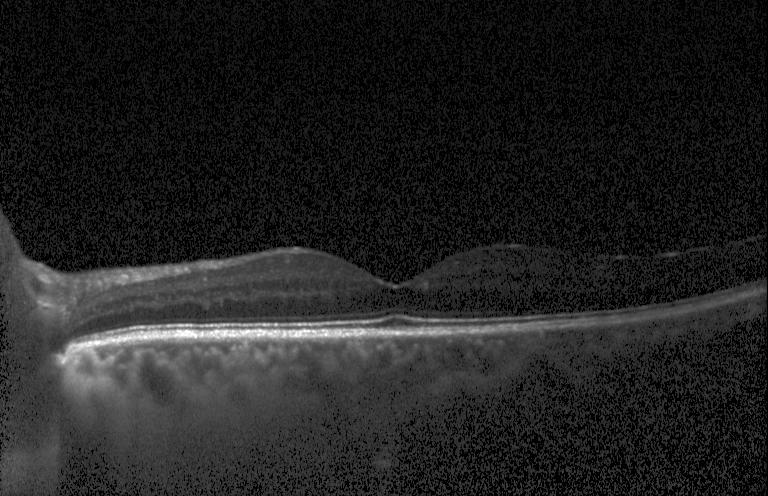
SD-OCT; centered on the fovea; OCT line scan
The scan shows no choroidal neovascularization, no diabetic macular edema, and no drusen.